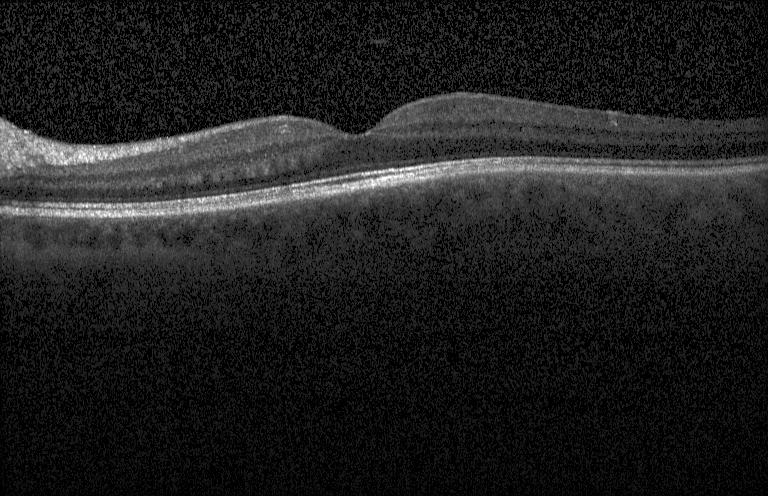
Instrument: Heidelberg Spectralis. Through the macula. Retinal OCT cross-section — Finding: no evidence of choroidal neovascularization, diabetic macular edema, or drusen.